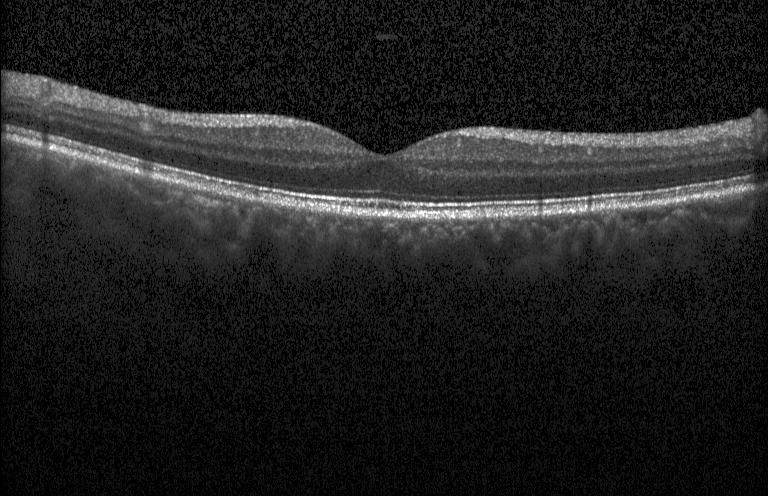 OCT B-scan. SD-OCT. Fovea-centered. Acquired on a Heidelberg Spectralis.
OCT finding: no choroidal neovascularization, diabetic macular edema, or drusen.